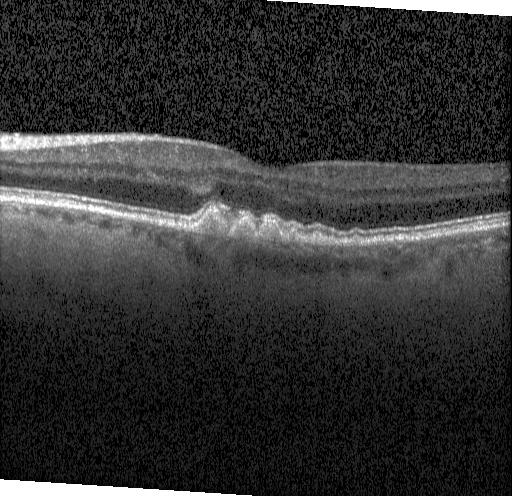
Impression: drusen.